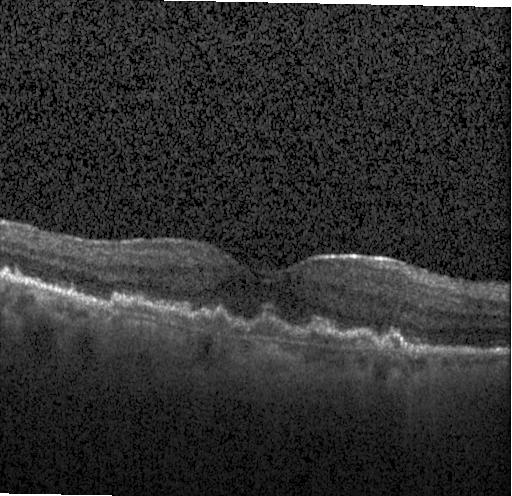

Choroidal neovascularization.